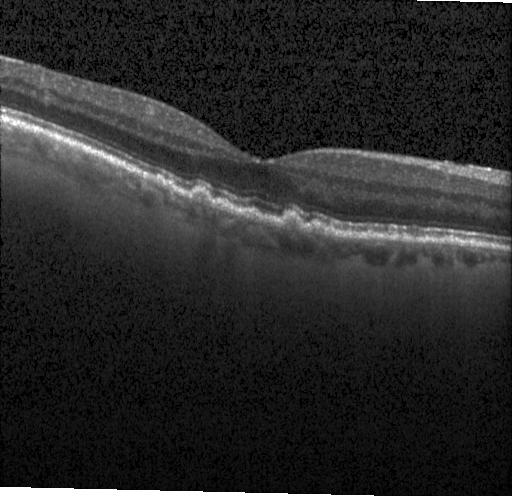 Horizontal scan through the fovea. Optical coherence tomography B-scan. The scan shows drusen.